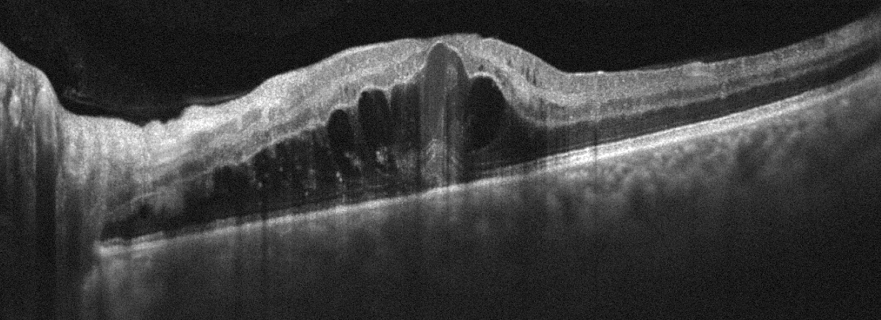

Fovea-centered. Retinal OCT B-scan. Acquired on an Optovue Avanti RTVue XR
Macular OCT: retinal vein occlusion.